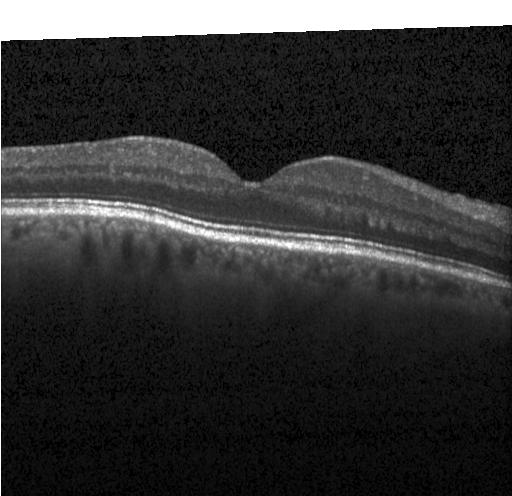

Retinal OCT cross-section showing neither CNV, DME, nor drusen.